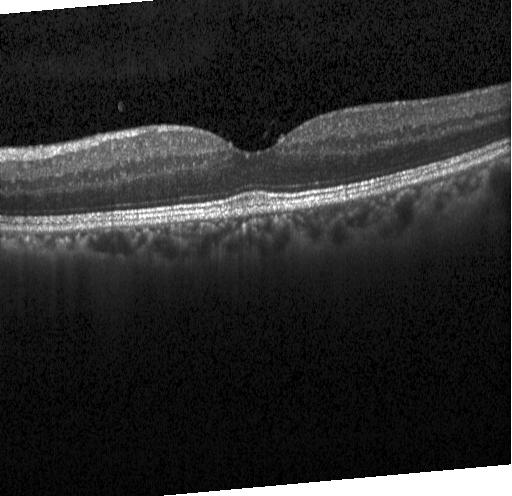

Macular OCT demonstrating no CNV, no DME, and no drusen.